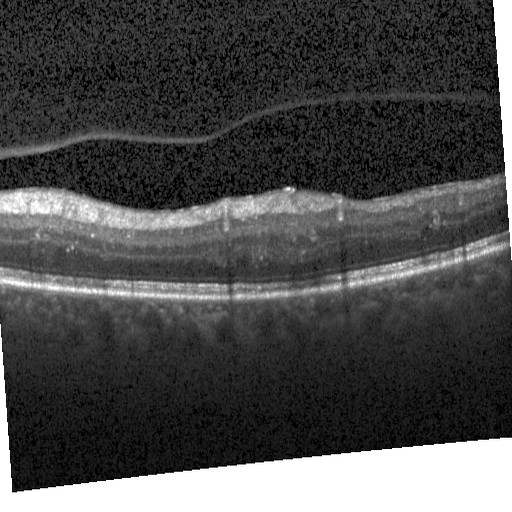
The scan shows diabetic macular edema.